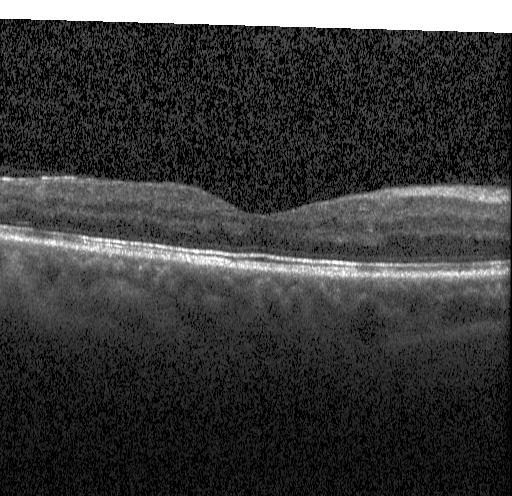 Heidelberg Spectralis, retinal OCT cross-section, macular scan
Macular OCT: no evidence of choroidal neovascularization, diabetic macular edema, or drusen.